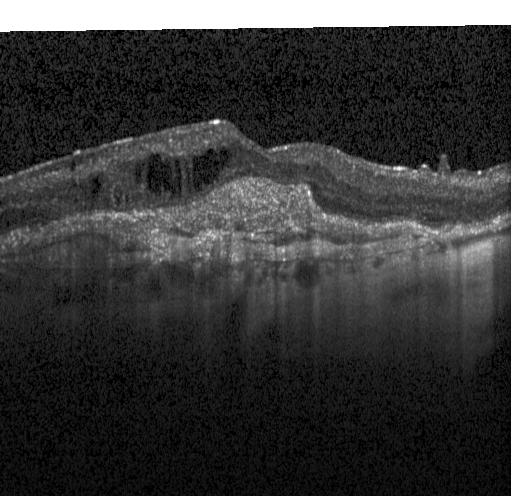

Diagnosis: a choroidal neovascular membrane.